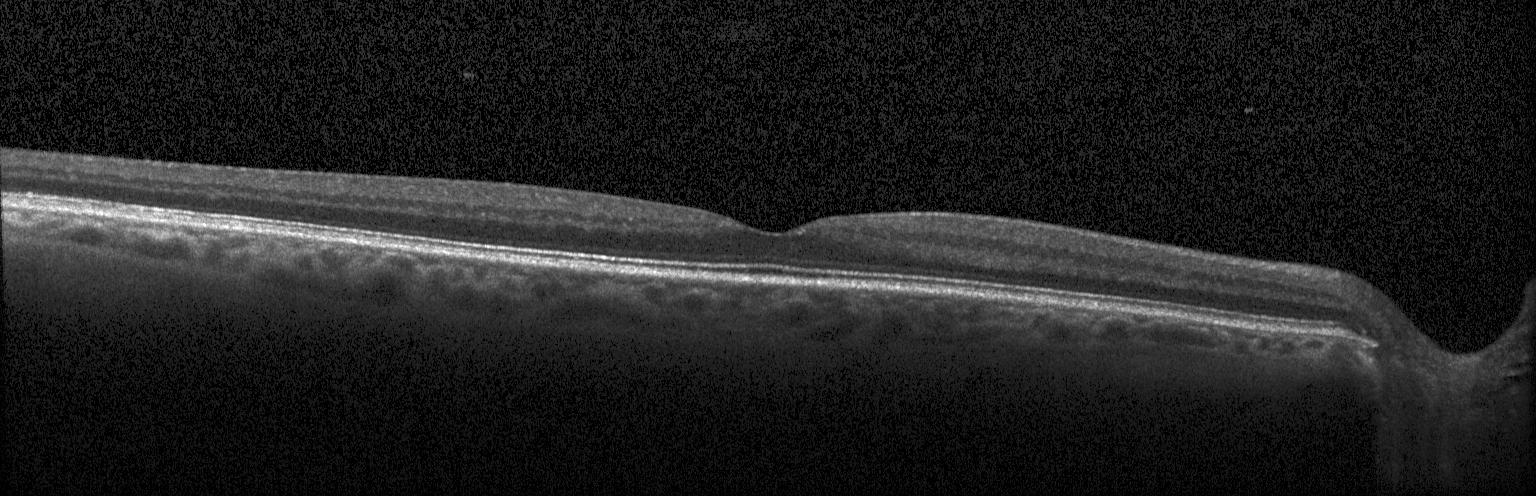
Instrument: Heidelberg Spectralis · through the macula · retinal OCT cross-section.
Macular OCT: no choroidal neovascularization, no diabetic macular edema, and no drusen.